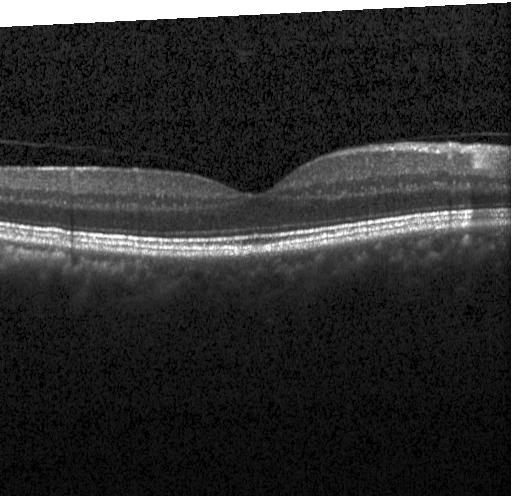
Heidelberg Spectralis OCT system; macular scan; optical coherence tomography B-scan; spectral-domain optical coherence tomography
Diagnosis: neither choroidal neovascularization, diabetic macular edema, nor drusen.